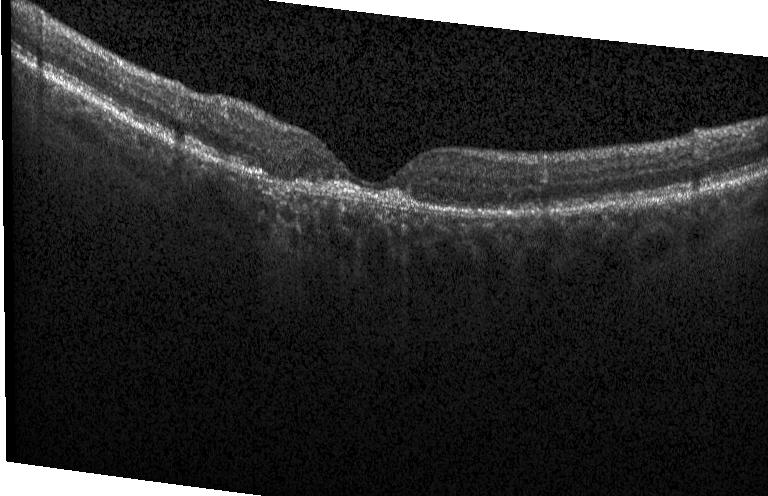 OCT B-scan, acquired on a Heidelberg Spectralis.
Assessment: a choroidal neovascular membrane.